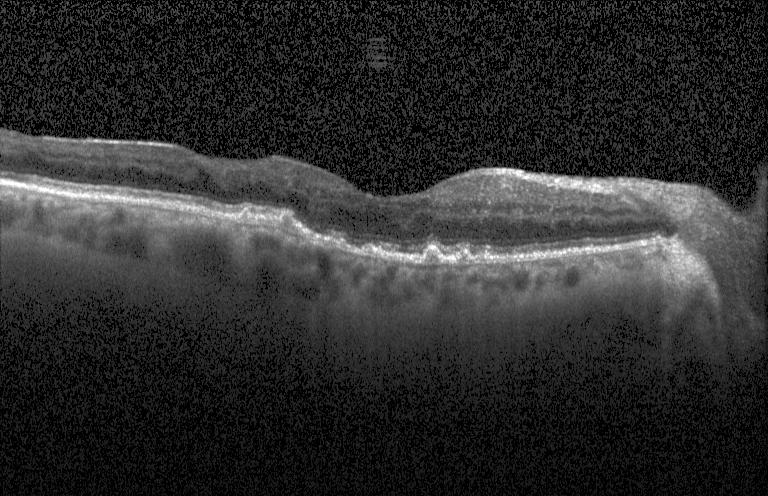 The scan shows multiple drusen.